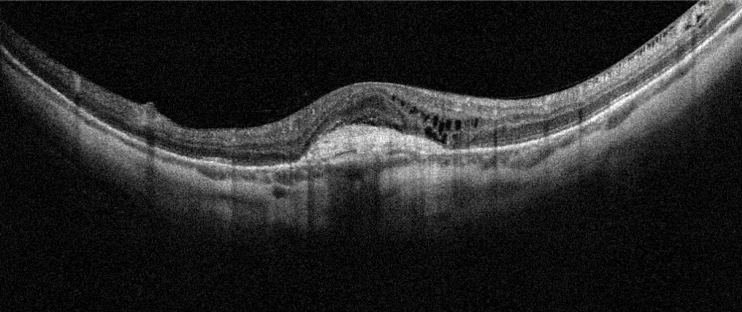 Macular OCT: AMD.